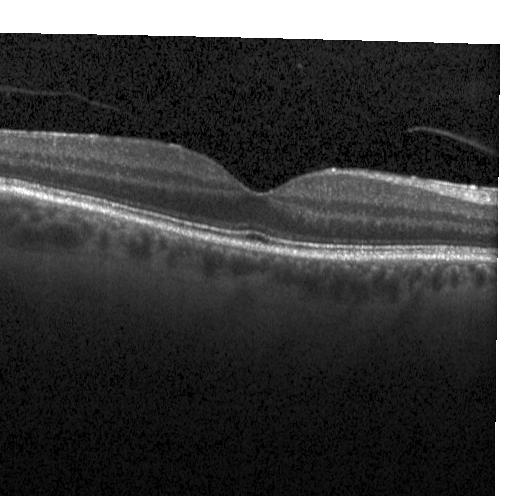

Centered on the fovea · retinal OCT B-scan · SD-OCT · Heidelberg Spectralis.
Diagnosis: no choroidal neovascularization, no diabetic macular edema, and no drusen.